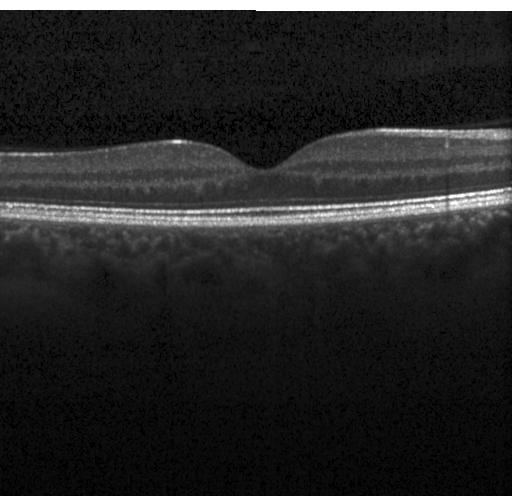
OCT B-scan.
The scan shows no evidence of CNV, DME, or drusen.